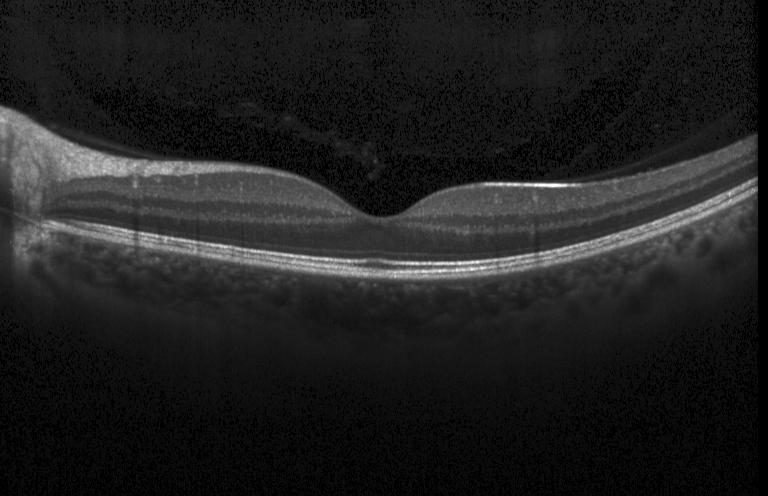 Horizontal scan through the fovea · optical coherence tomography scan · SD-OCT — The scan shows no choroidal neovascularization, diabetic macular edema, or drusen.